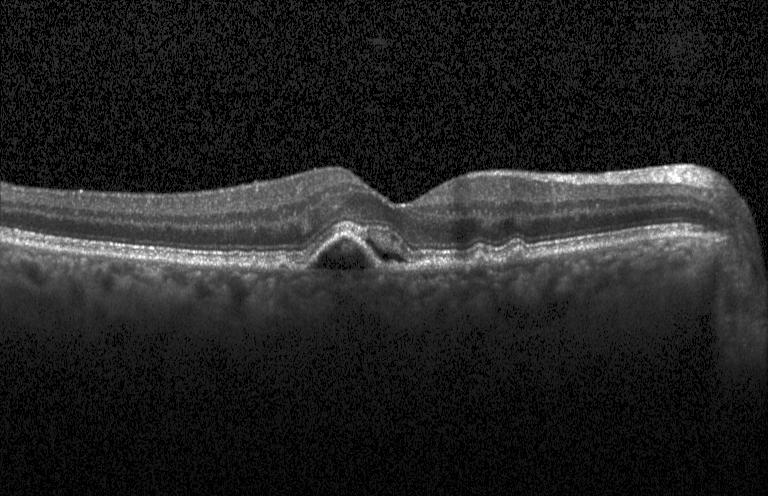

This B-scan demonstrates choroidal neovascularization (CNV).